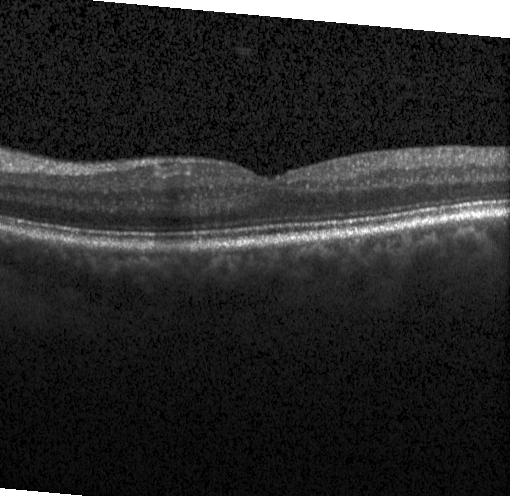
Heidelberg Spectralis OCT system; OCT B-scan; spectral-domain optical coherence tomography. Assessment: no choroidal neovascularization, diabetic macular edema, or drusen.